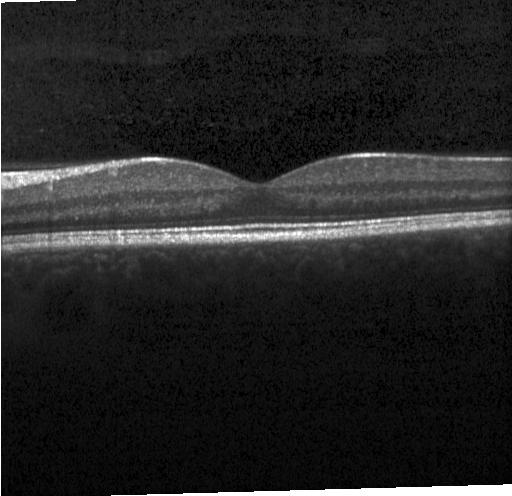
Heidelberg Spectralis OCT system; through the macula; optical coherence tomography scan. Diagnosis: no choroidal neovascularization, no diabetic macular edema, and no drusen.